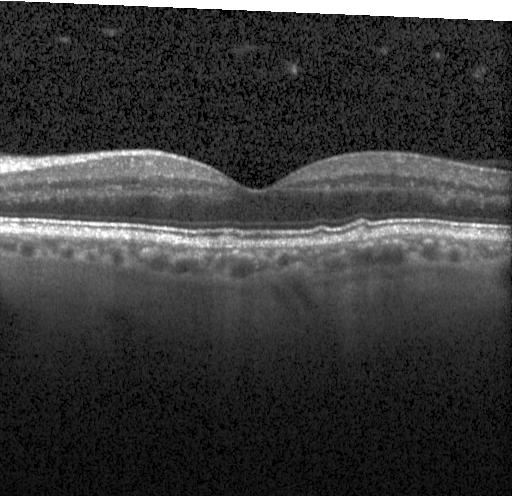
OCT B-scan. Finding: neither CNV, DME, nor drusen.